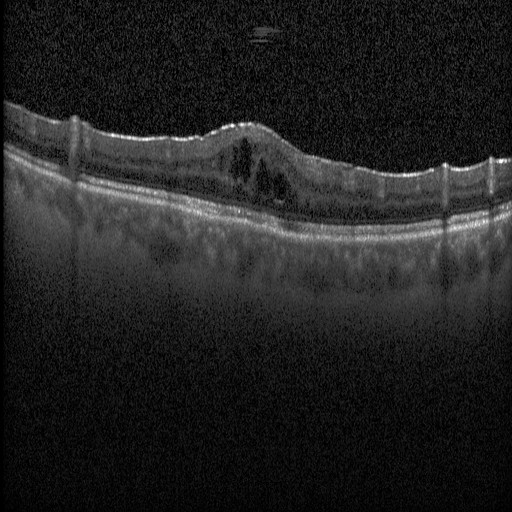 OCT B-scan, SD-OCT — Impression: DME.